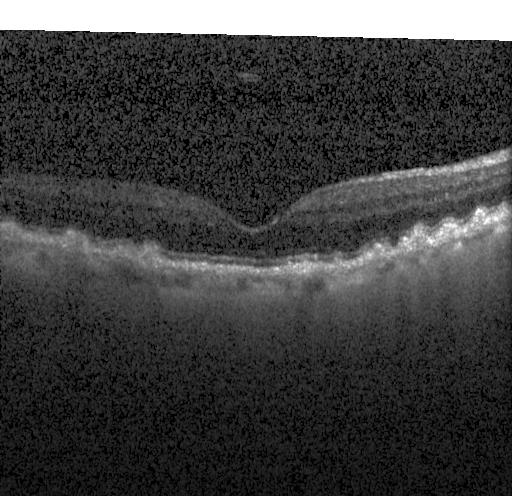
Assessment: sub-RPE drusenoid deposits.